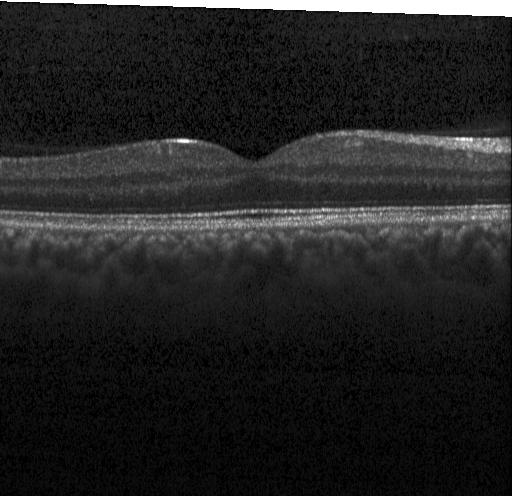
Horizontal scan through the fovea; OCT B-scan; Heidelberg Spectralis OCT system — Assessment: no evidence of choroidal neovascularization, diabetic macular edema, or drusen.